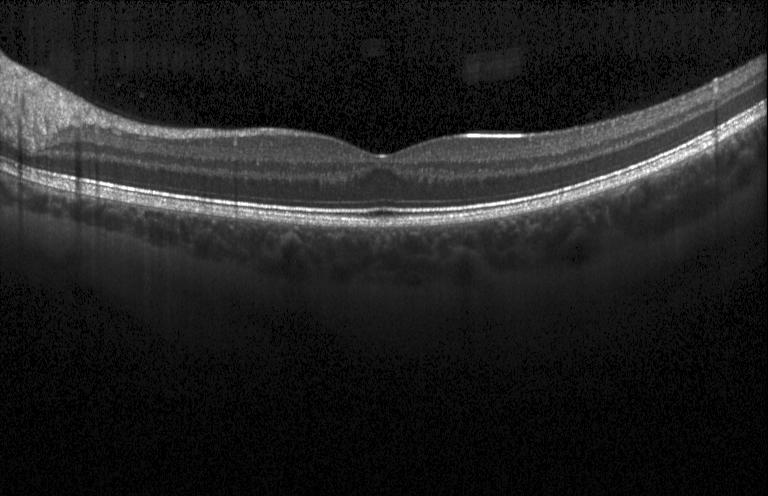 Macular OCT: no evidence of CNV, DME, or drusen.